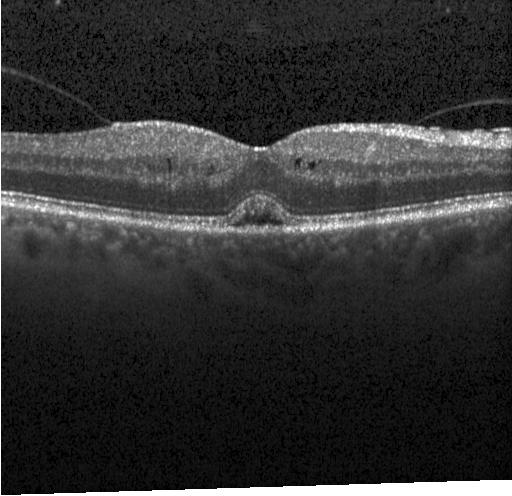

OCT line scan · acquired on a Heidelberg Spectralis — Finding: diabetic macular edema.